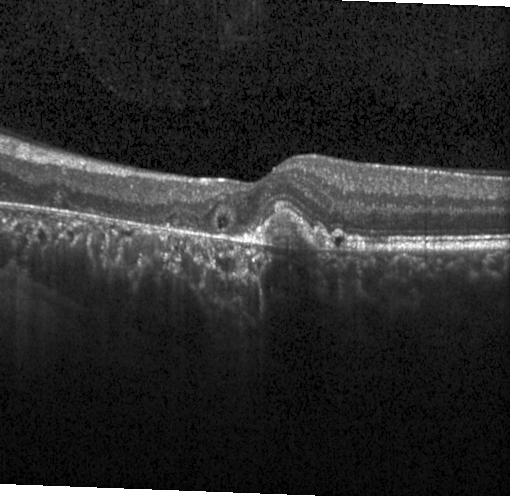

OCT B-scan showing CNV.